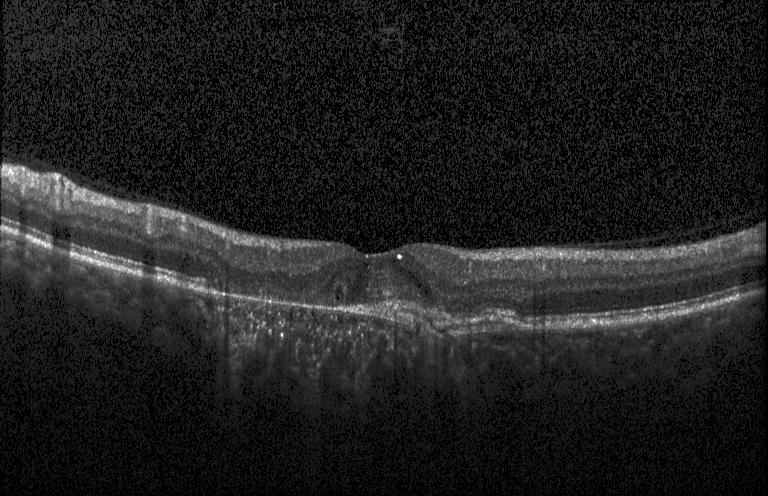
OCT finding: a choroidal neovascular membrane.